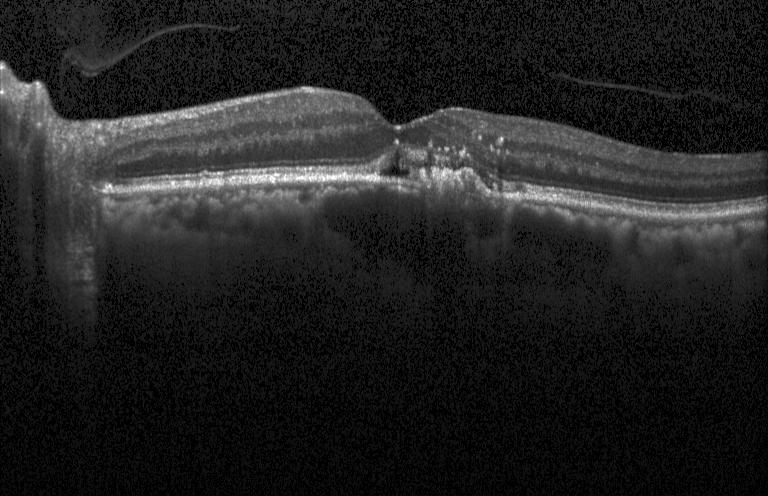

Impression: a choroidal neovascular membrane.